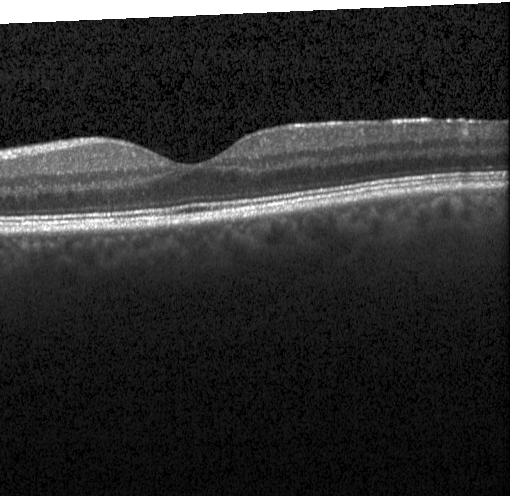 Through the macula; spectral-domain OCT; OCT B-scan. Impression: neither choroidal neovascularization, diabetic macular edema, nor drusen.